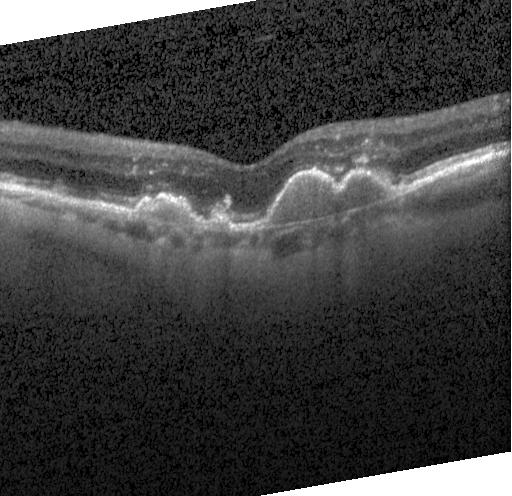 OCT B-scan.
Dx: a choroidal neovascular membrane.